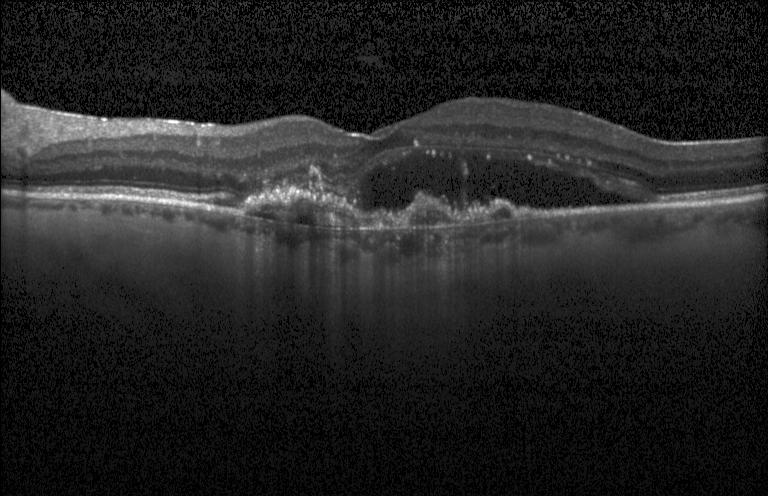
OCT B-scan; spectral-domain OCT; through the macula — Diagnosis: choroidal neovascularization (CNV).